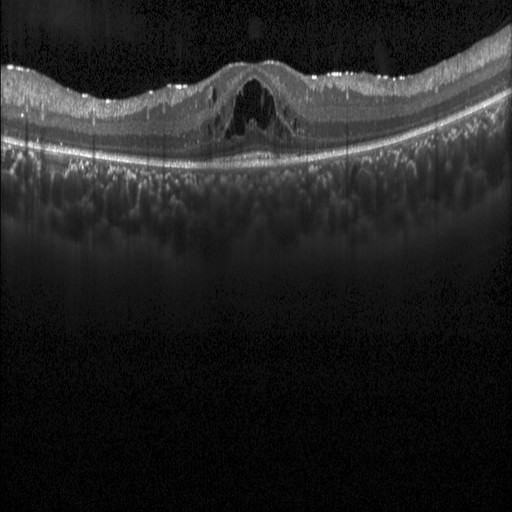

Optical coherence tomography B-scan
Diagnosis: diabetic macular edema.